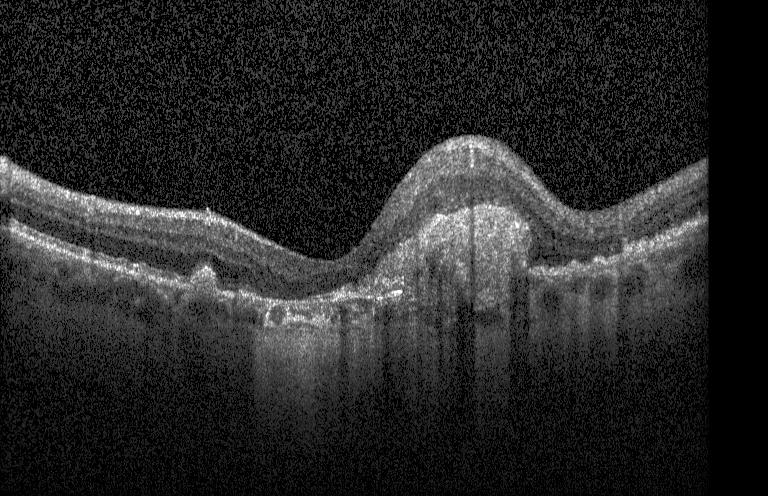 Spectral-domain OCT B-scan: choroidal neovascularization (CNV).